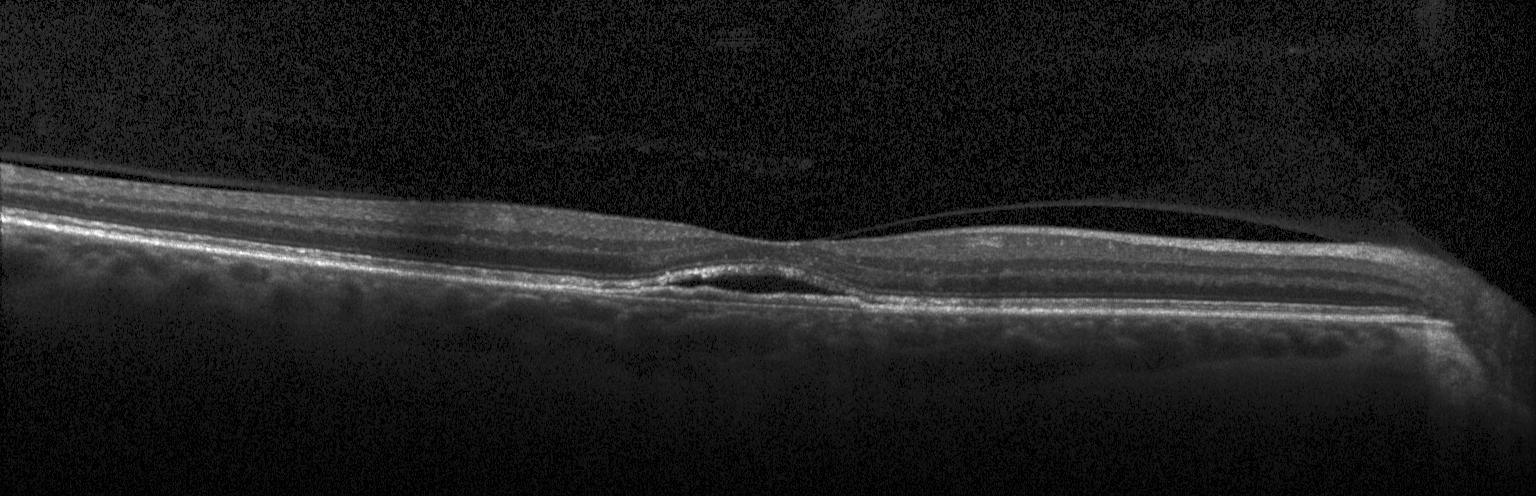 Instrument: Heidelberg Spectralis, retinal OCT cross-section, SD-OCT, macular scan — Impression: CNV.